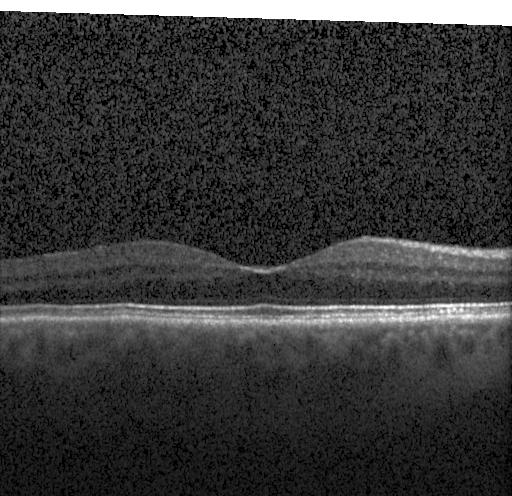
Heidelberg Spectralis OCT system, retinal OCT B-scan. The scan shows neither CNV, DME, nor drusen.